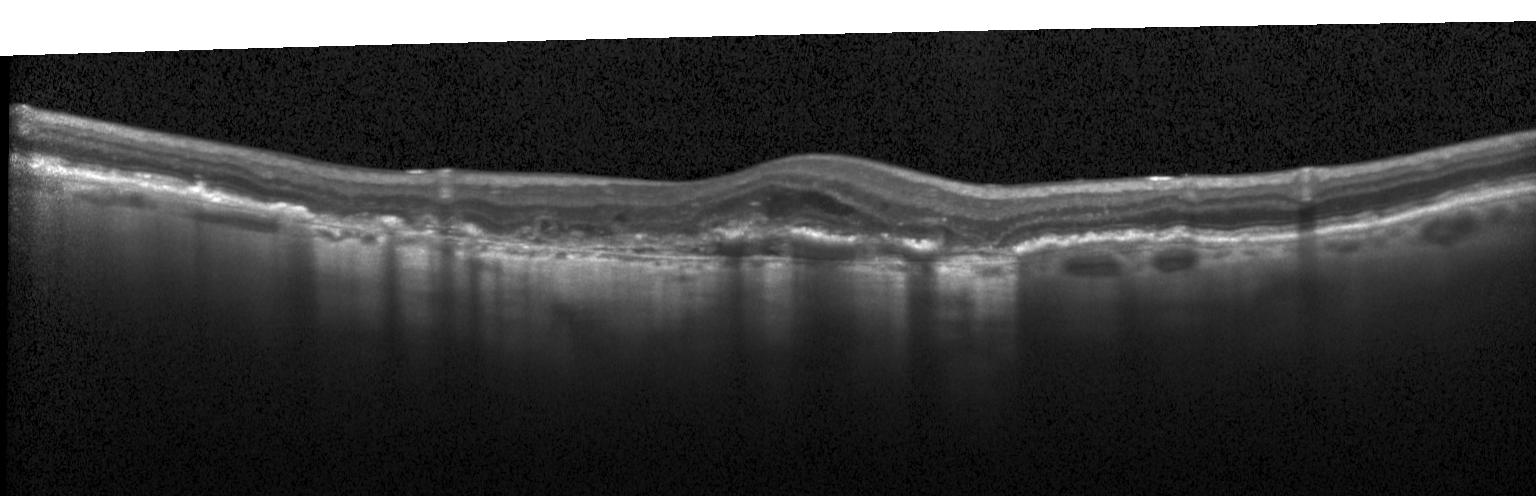 Optical coherence tomography scan
Assessment: choroidal neovascularization (CNV).